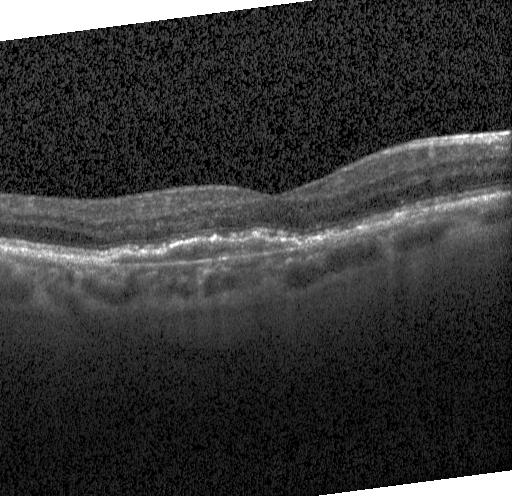
Retinal OCT cross-section.
OCT finding: CNV.